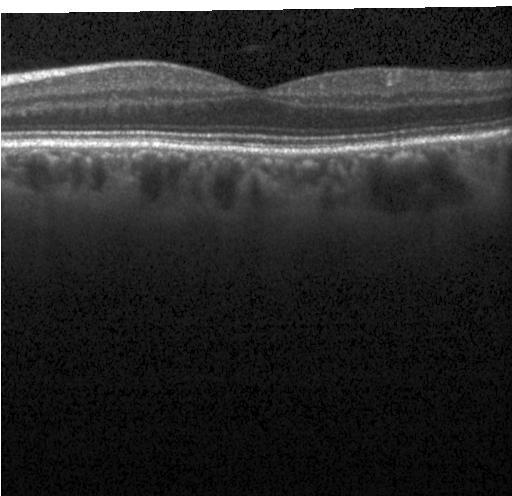
Optical coherence tomography B-scan. Heidelberg Spectralis OCT system. Macular scan. SD-OCT
Diagnosis: no choroidal neovascularization, diabetic macular edema, or drusen.